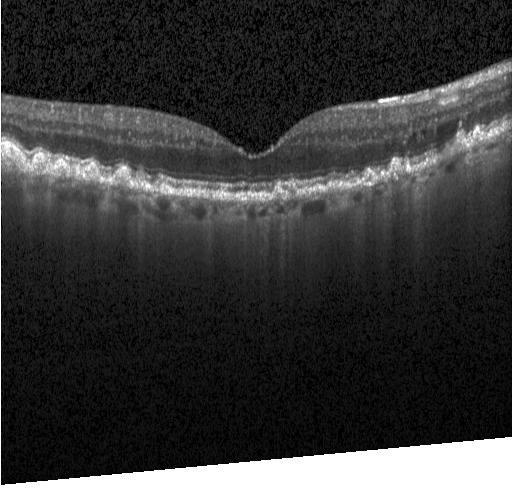
Dx: sub-RPE drusenoid deposits.